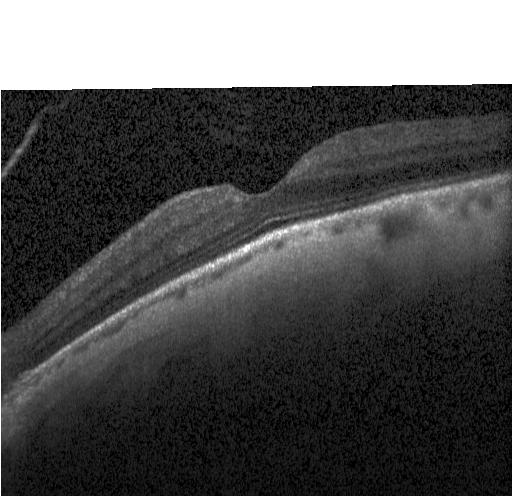

Impression: neither choroidal neovascularization, diabetic macular edema, nor drusen.